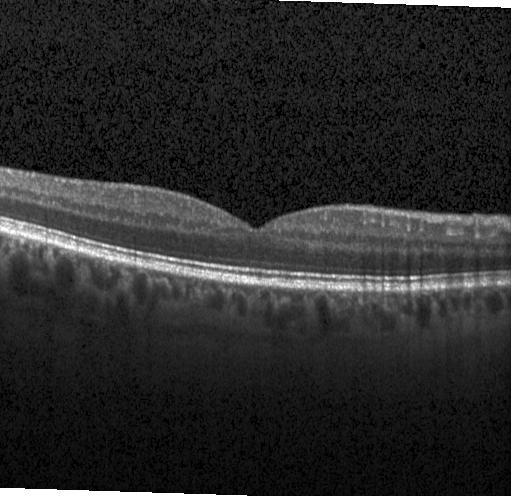
Retinal OCT cross-section, Heidelberg Spectralis OCT system
Dx: no CNV, no DME, and no drusen.